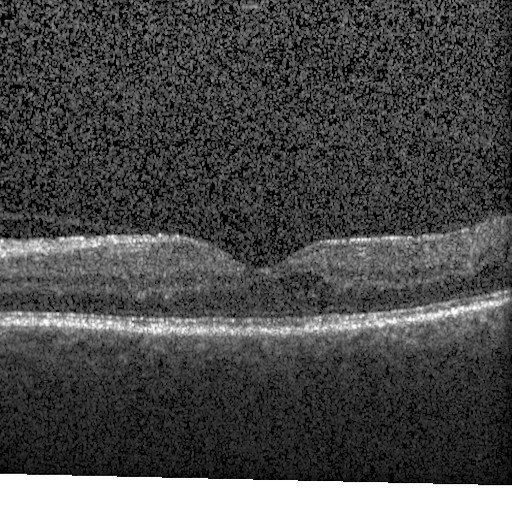 Optical coherence tomography scan — Dx: diabetic macular edema.